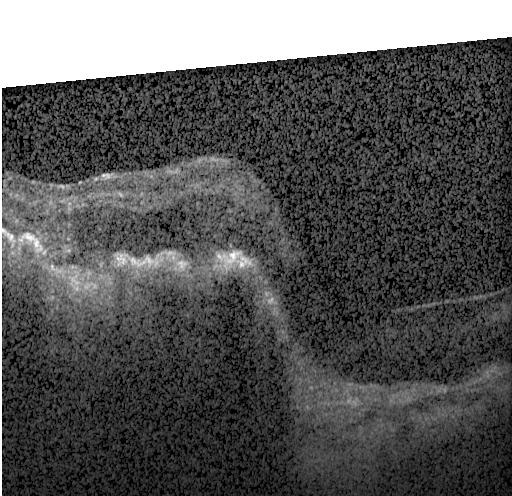
Finding: a choroidal neovascular membrane.